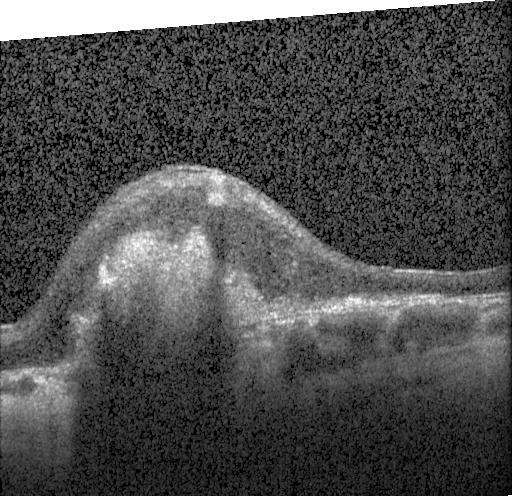

Choroidal neovascularization.